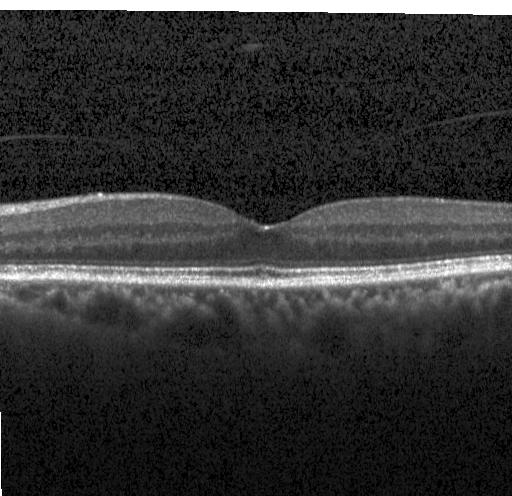 Optical coherence tomography B-scan; fovea-centered; SD-OCT.
Macular OCT: no choroidal neovascularization, no diabetic macular edema, and no drusen.